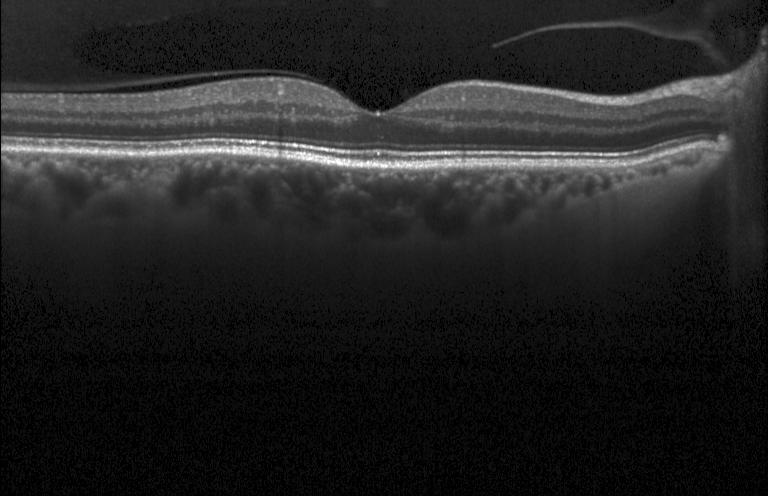
The scan shows no evidence of CNV, DME, or drusen.